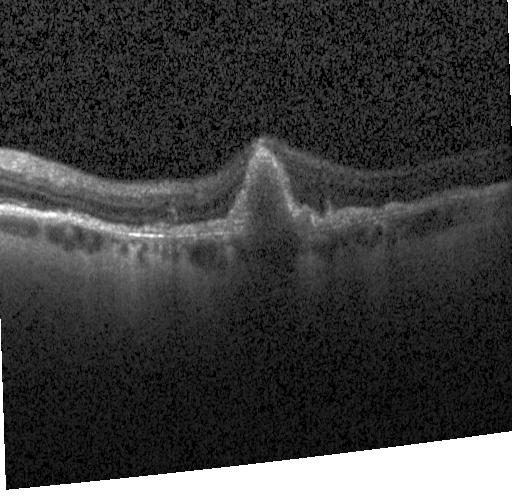

Centered on the fovea; Heidelberg Spectralis; OCT B-scan; spectral-domain OCT.
Impression: choroidal neovascularization (CNV).